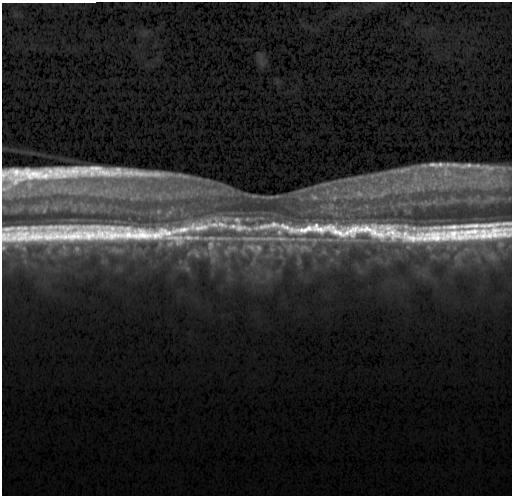

Retinal OCT cross-section · spectral-domain optical coherence tomography · Heidelberg Spectralis OCT system.
Diagnosis: CNV.